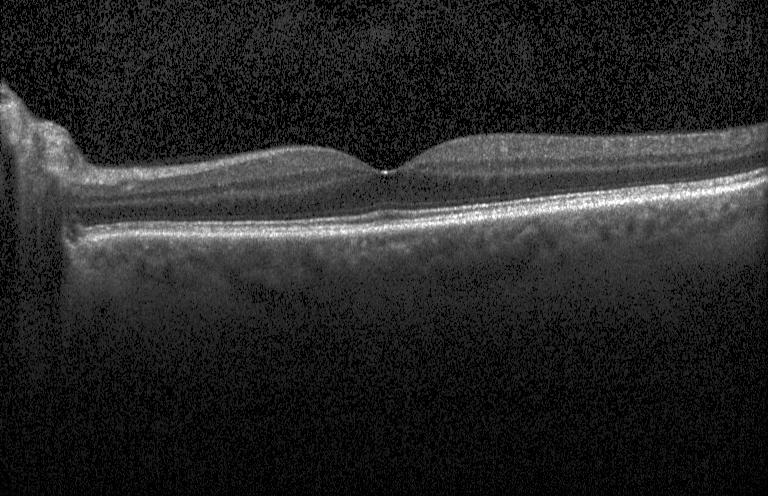

Heidelberg Spectralis OCT system; macular scan; retinal OCT cross-section — Diagnosis: no choroidal neovascularization, diabetic macular edema, or drusen.